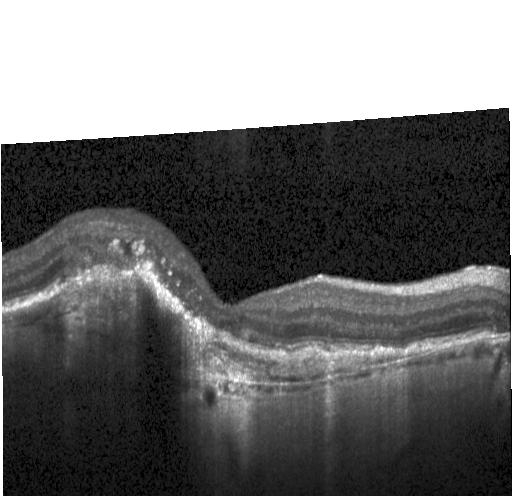
OCT B-scan showing choroidal neovascularization.